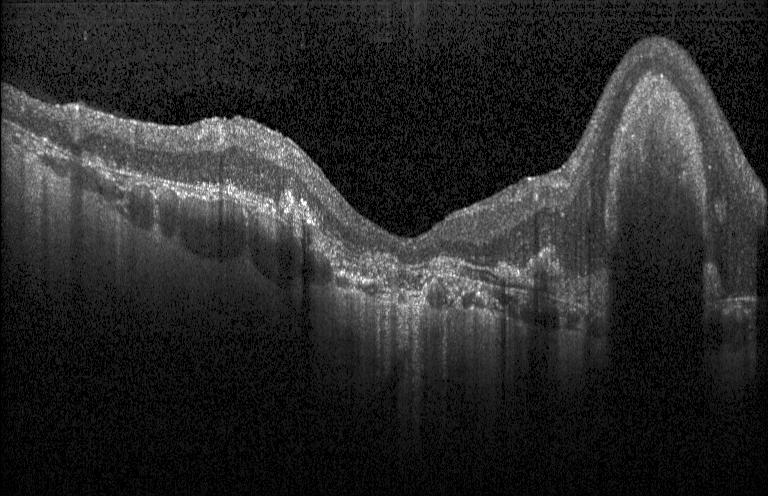
SD-OCT. Retinal OCT B-scan.
Diagnosis: CNV.